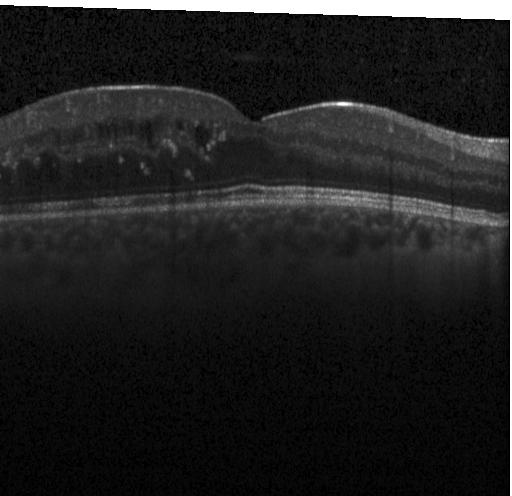

Optical coherence tomography scan.
Finding: DME.